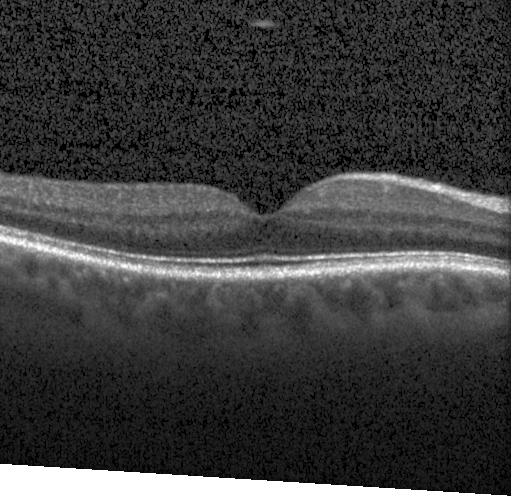 OCT line scan. Impression: no evidence of choroidal neovascularization, diabetic macular edema, or drusen.